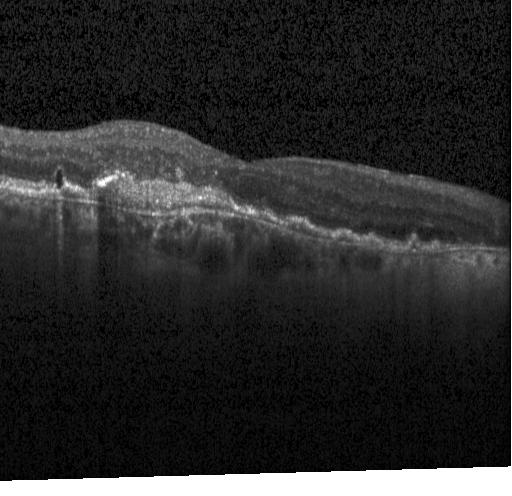

Retinal OCT B-scan. Diagnosis: a choroidal neovascular membrane.